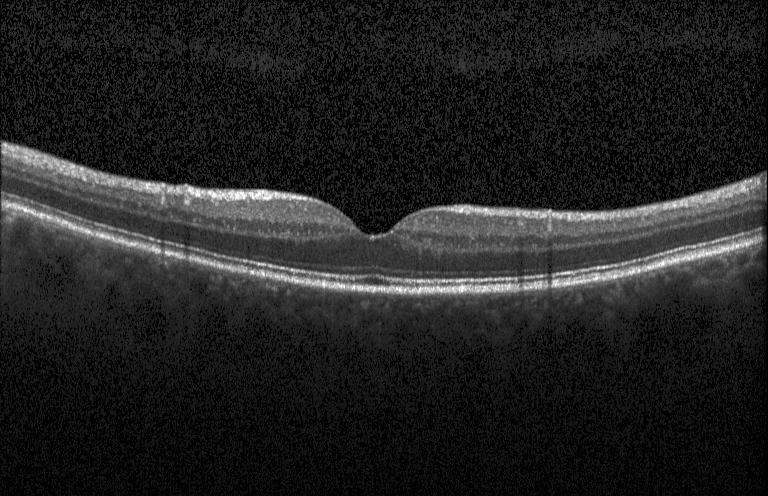 Retinal OCT cross-section.
Impression: no CNV, no DME, and no drusen.